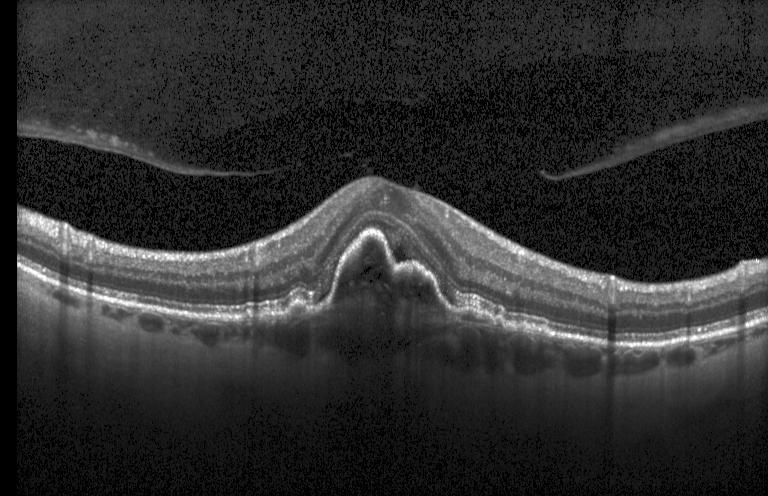

Diagnosis: CNV.